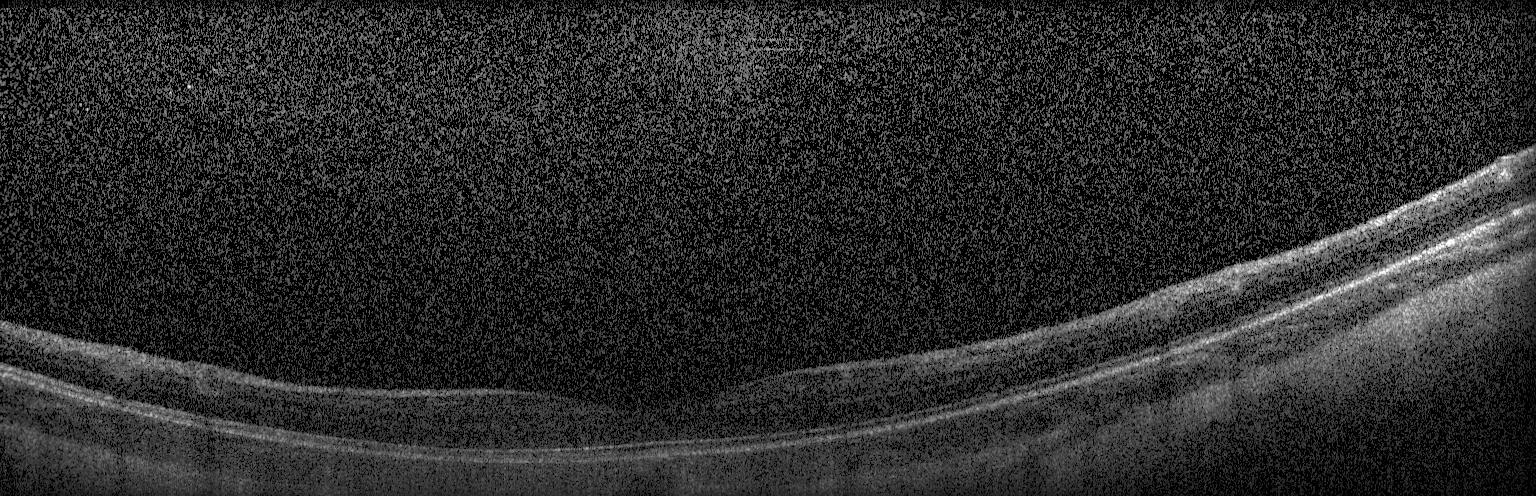
OCT line scan. Finding: no choroidal neovascularization, no diabetic macular edema, and no drusen.